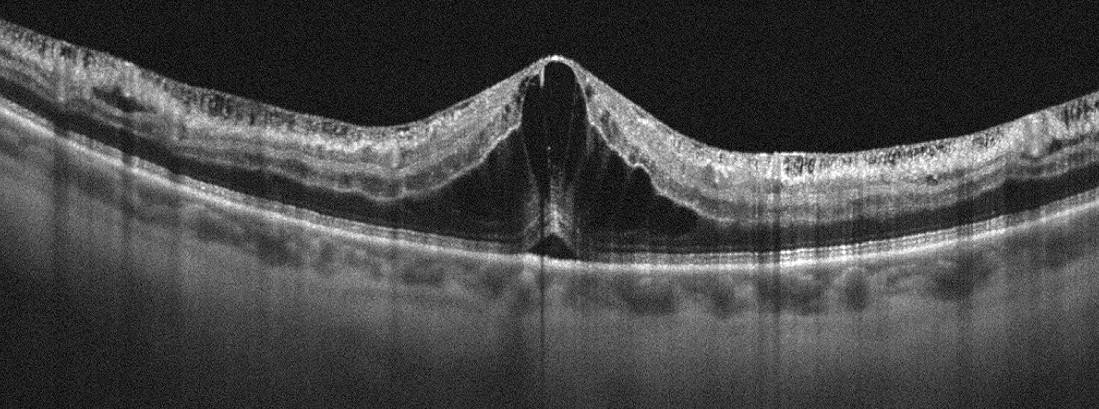

Macular scan. OCT line scan. Instrument: Optovue Avanti RTVue XR. Diagnosis: RVO.